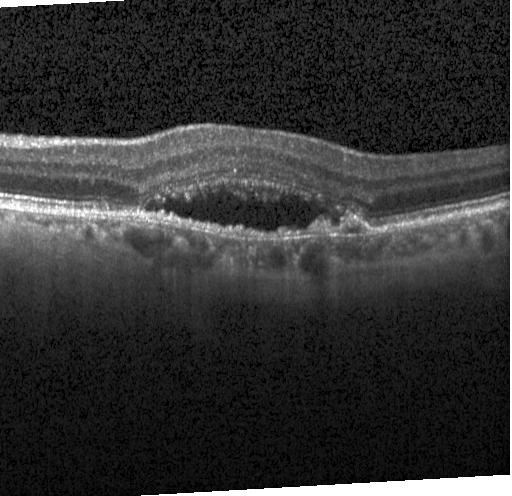

Retinal OCT cross-section showing CNV.